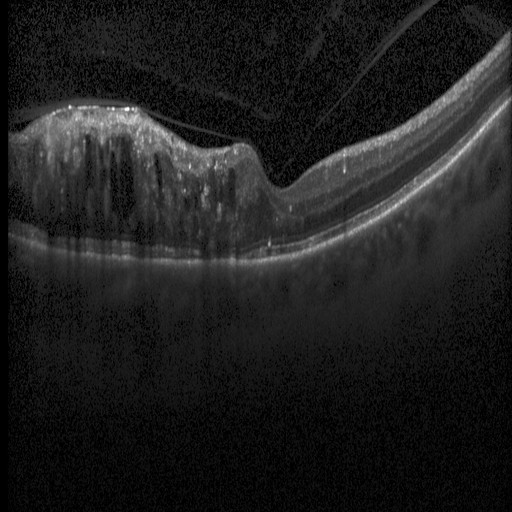 Impression: diabetic macular edema (DME).